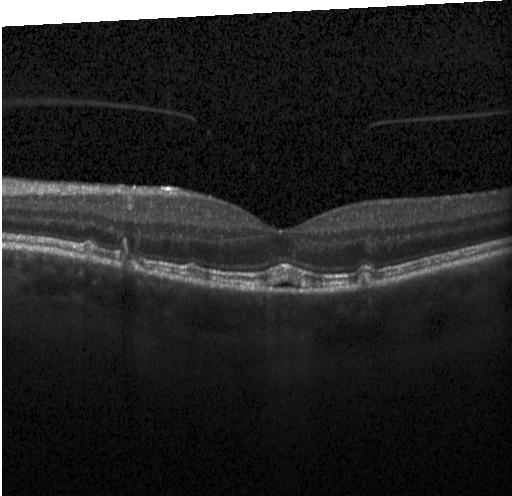 Retinal OCT B-scan, through the macula, spectral-domain OCT — Drusen.